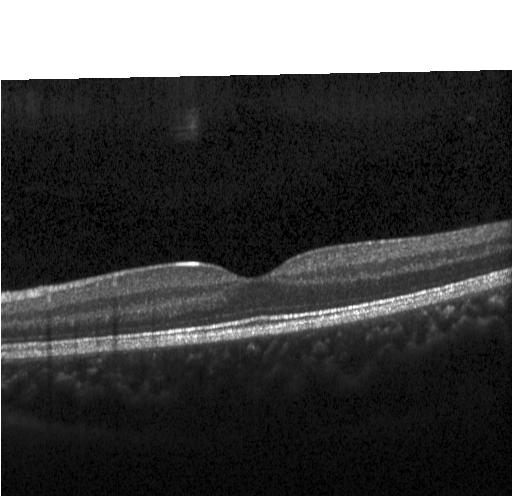 Heidelberg Spectralis · OCT B-scan · spectral-domain OCT
Diagnosis: neither choroidal neovascularization, diabetic macular edema, nor drusen.